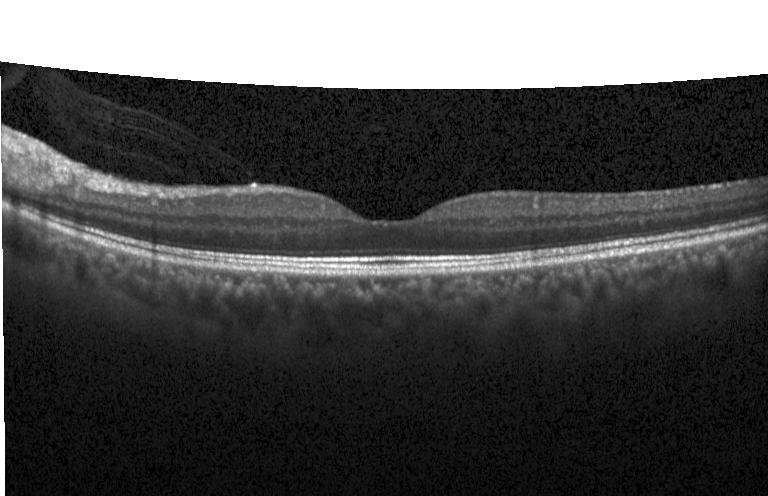

Heidelberg Spectralis OCT system; macular scan; SD-OCT; optical coherence tomography B-scan
Impression: neither choroidal neovascularization, diabetic macular edema, nor drusen.